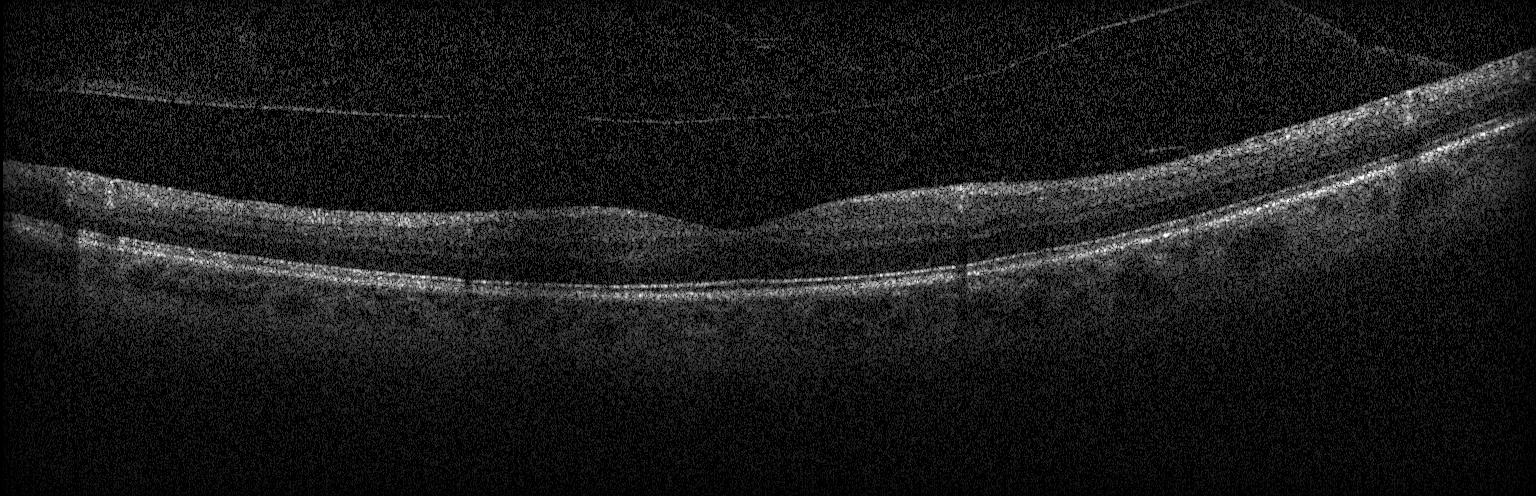 Centered on the fovea; optical coherence tomography B-scan
Macular OCT: no evidence of choroidal neovascularization, diabetic macular edema, or drusen.